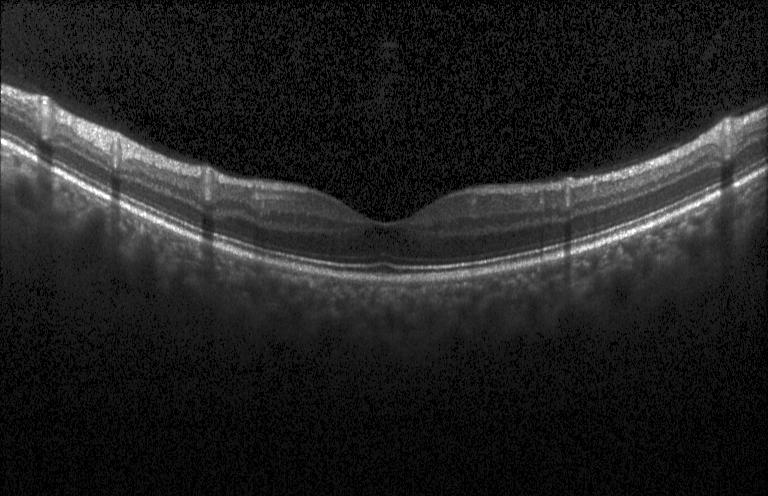
SD-OCT; retinal OCT cross-section; macular scan — Impression: no evidence of choroidal neovascularization, diabetic macular edema, or drusen.